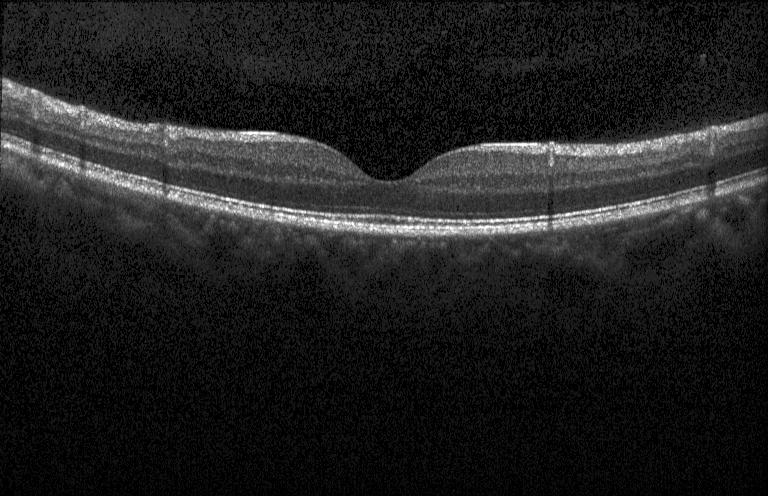

OCT B-scan showing no choroidal neovascularization, no diabetic macular edema, and no drusen.